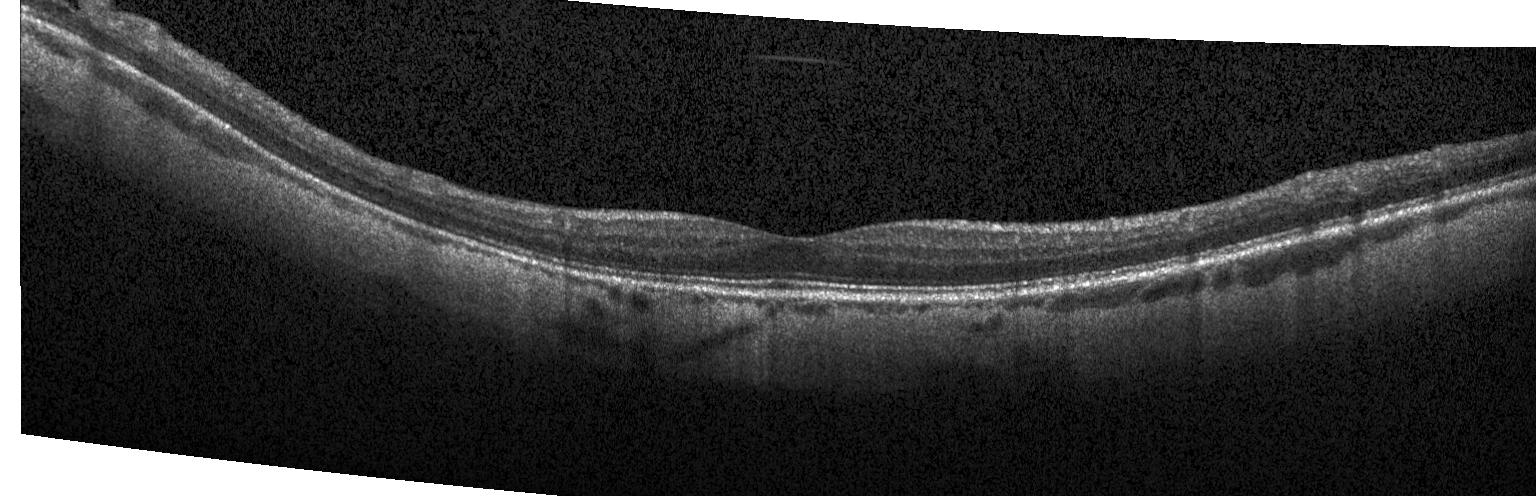
Macular OCT: no CNV, no DME, and no drusen.